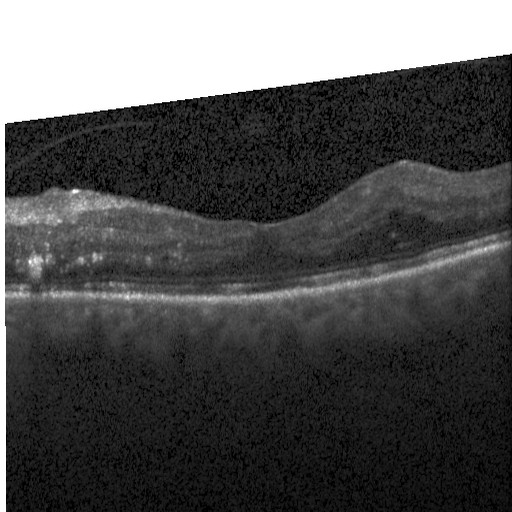

Dx: diabetic macular edema (DME).